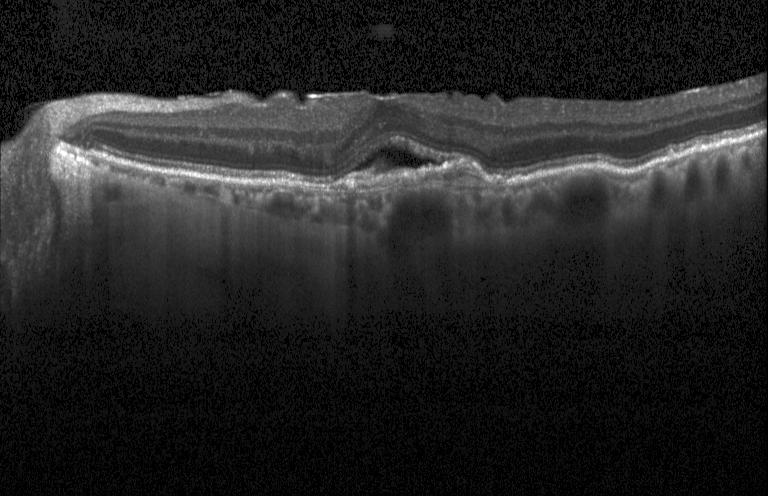

SD-OCT. Optical coherence tomography B-scan
Assessment: a choroidal neovascular membrane.